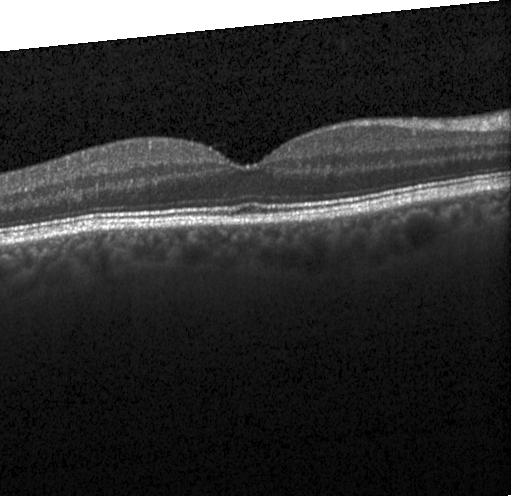

SD-OCT. Optical coherence tomography scan. Dx: no evidence of choroidal neovascularization, diabetic macular edema, or drusen.